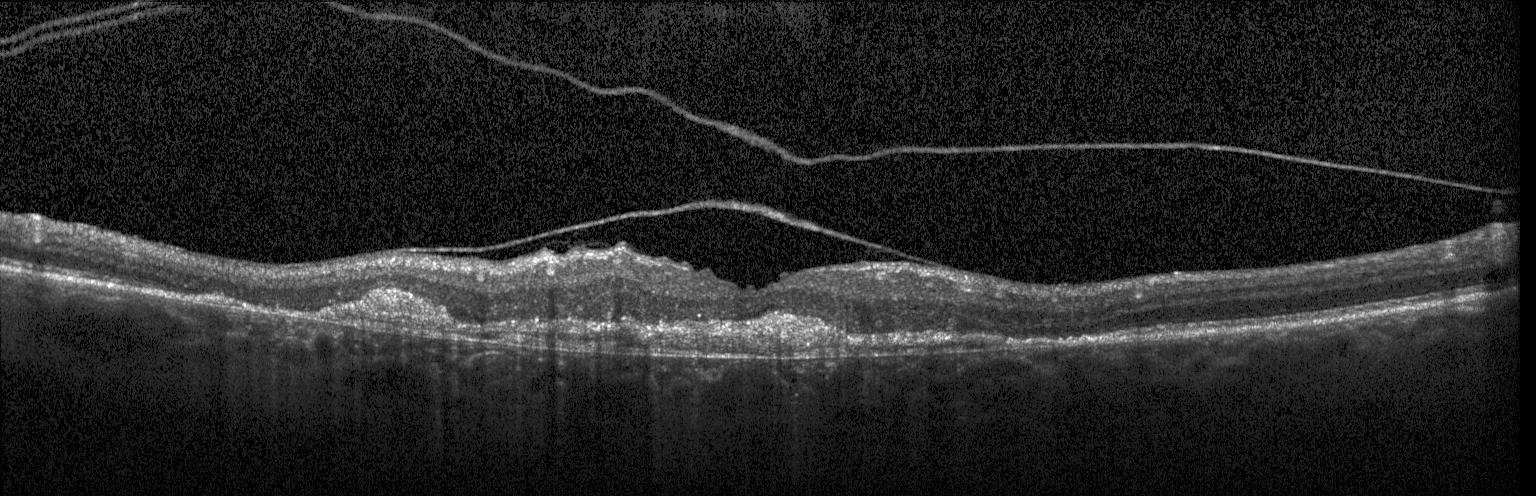 The scan shows a choroidal neovascular membrane.